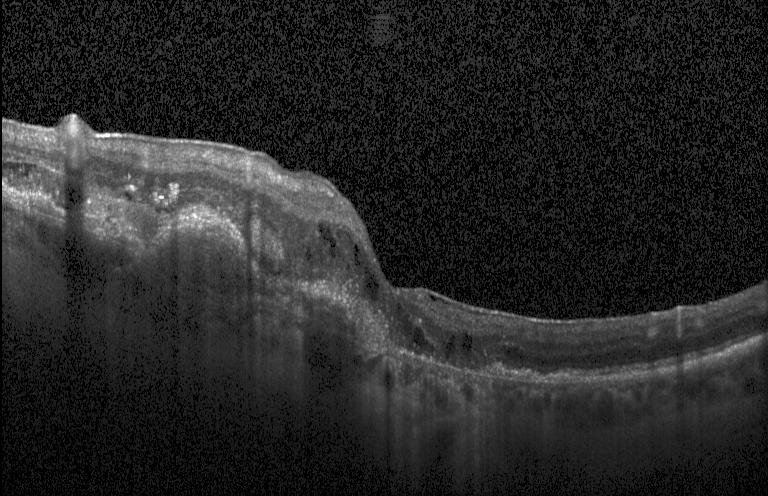 OCT finding: choroidal neovascularization (CNV).